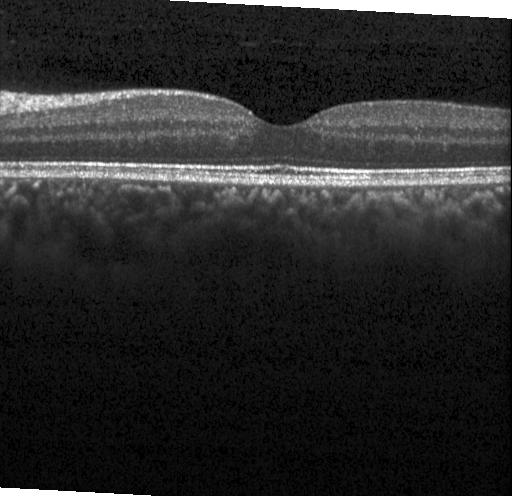 Spectral-domain OCT, instrument: Heidelberg Spectralis, OCT B-scan. Dx: no choroidal neovascularization, no diabetic macular edema, and no drusen.